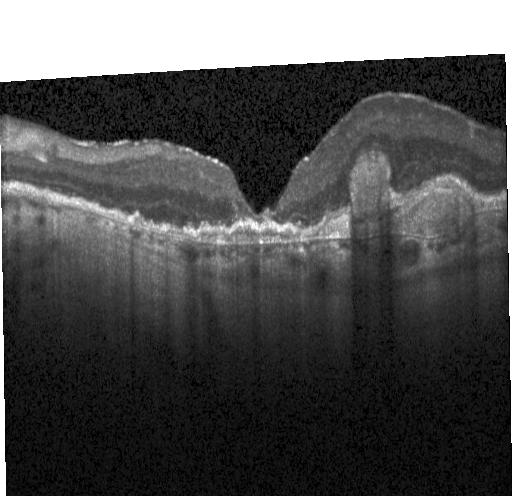
Impression: choroidal neovascularization (CNV).